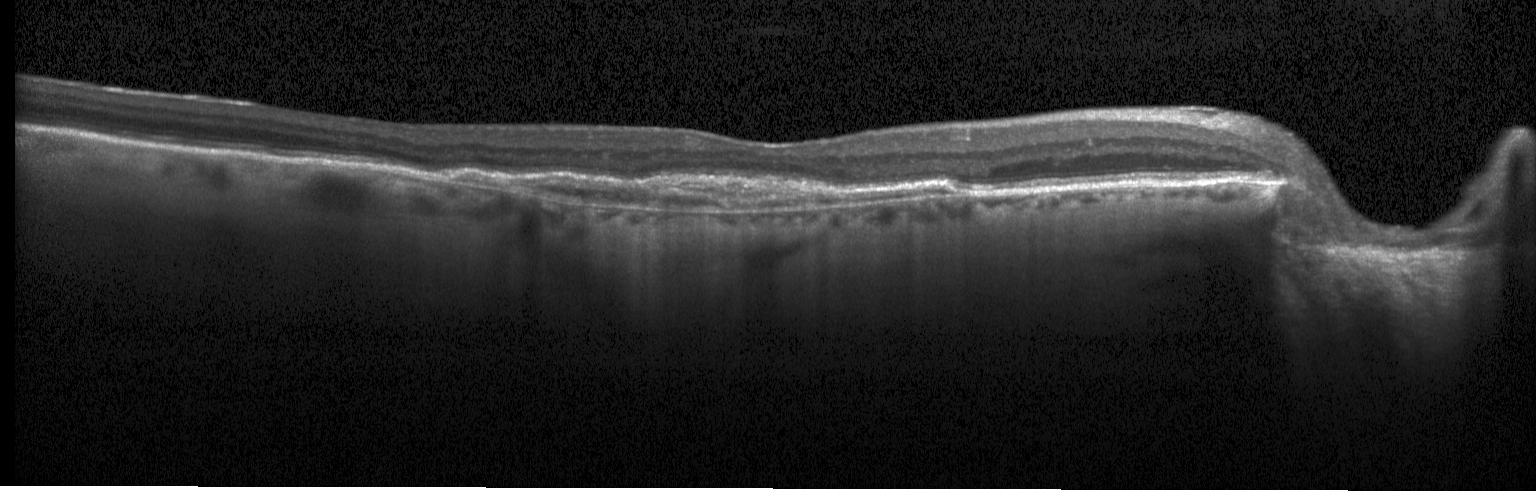
Retinal OCT cross-section. Horizontal scan through the fovea. Heidelberg Spectralis OCT system.
Assessment: choroidal neovascularization.